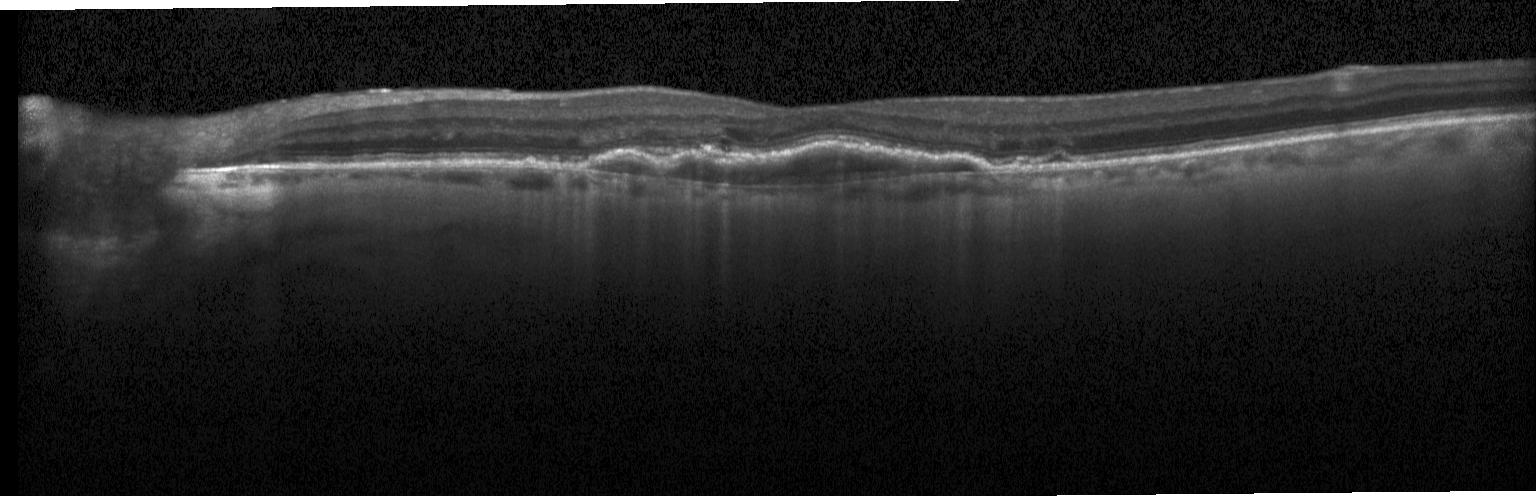
Retinal OCT cross-section
Dx: a choroidal neovascular membrane.